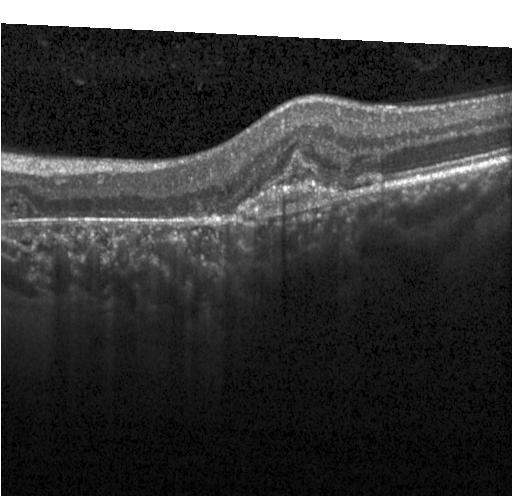

Diagnosis: a choroidal neovascular membrane.